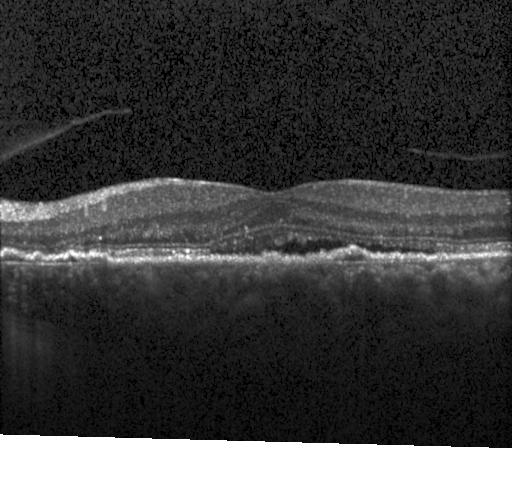
Impression: choroidal neovascularization (CNV).